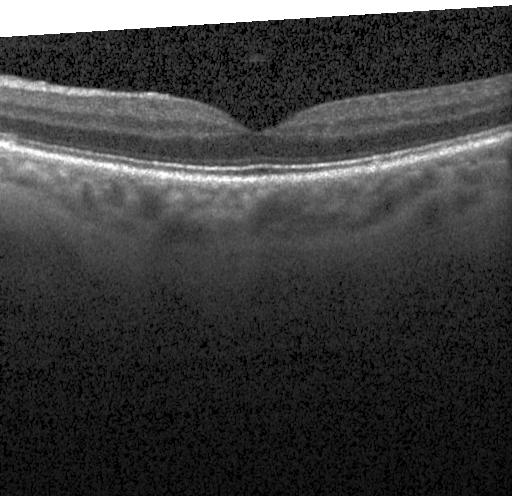

OCT B-scan · instrument: Heidelberg Spectralis · fovea-centered · SD-OCT — Diagnosis: neither CNV, DME, nor drusen.